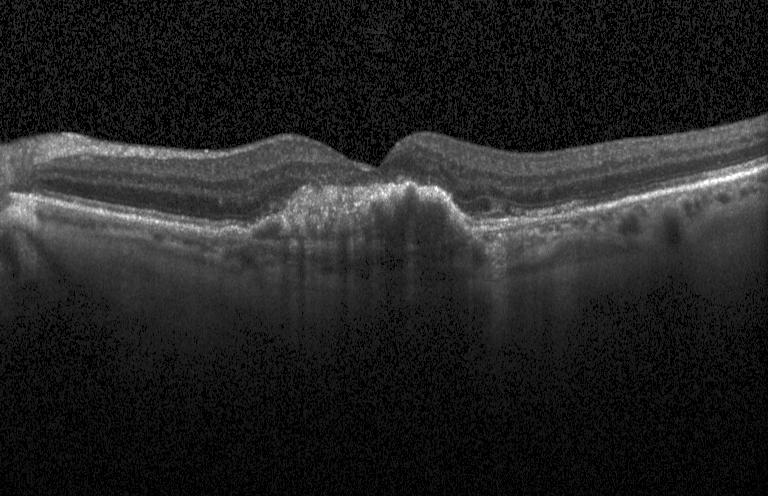

Retinal OCT cross-section. Through the macula
Finding: choroidal neovascularization.